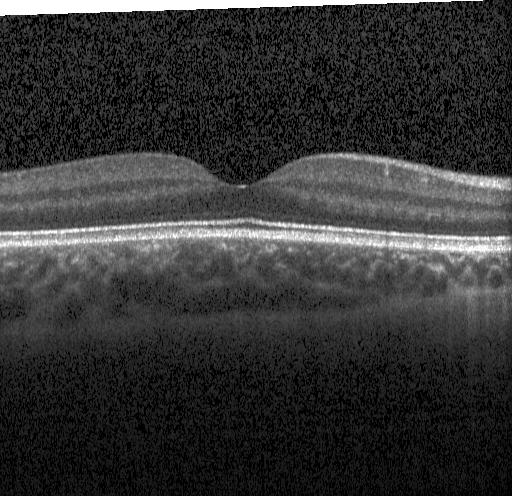

Centered on the fovea; OCT B-scan; instrument: Heidelberg Spectralis
Assessment: no choroidal neovascularization, no diabetic macular edema, and no drusen.